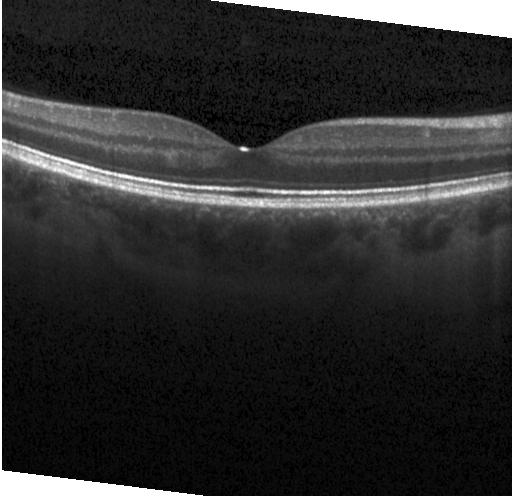

Macular OCT: no CNV, DME, or drusen.